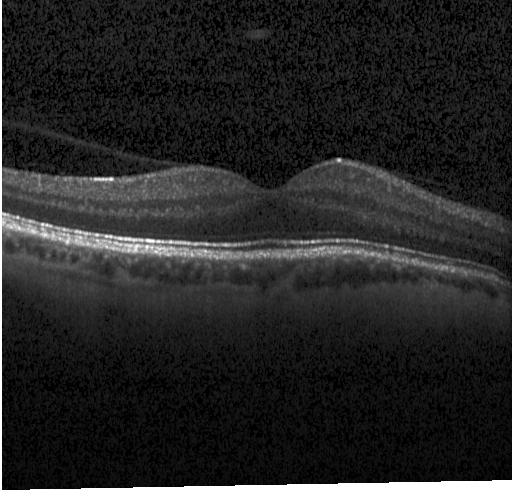
Diagnosis: neither CNV, DME, nor drusen.